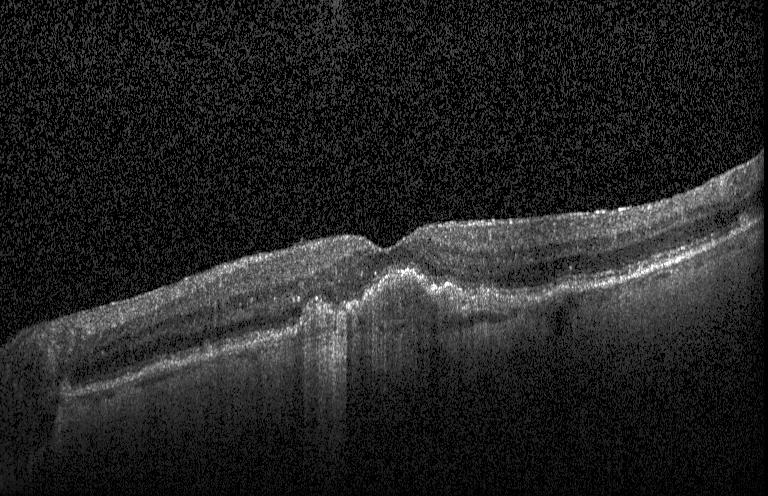 OCT finding: a choroidal neovascular membrane.